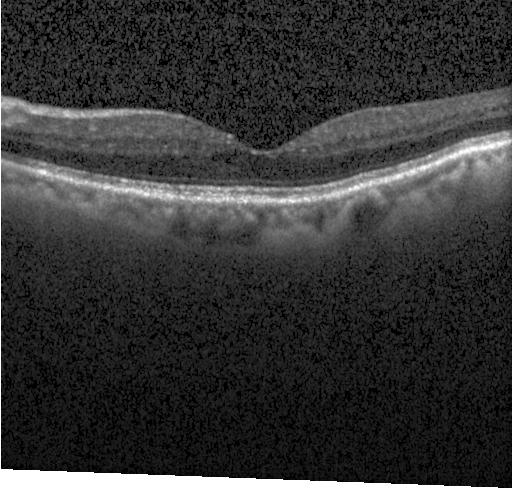 OCT finding: no evidence of choroidal neovascularization, diabetic macular edema, or drusen.